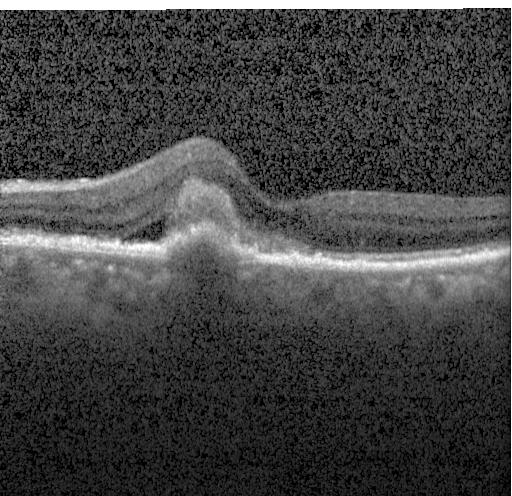
Acquired on a Heidelberg Spectralis. Retinal OCT cross-section. Spectral-domain optical coherence tomography — Finding: a choroidal neovascular membrane.